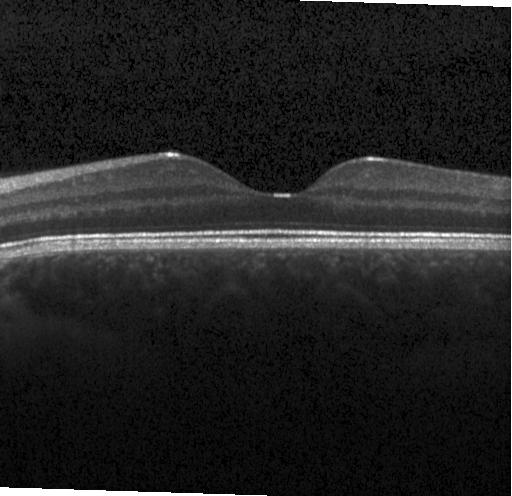 OCT scan showing no CNV, no DME, and no drusen.